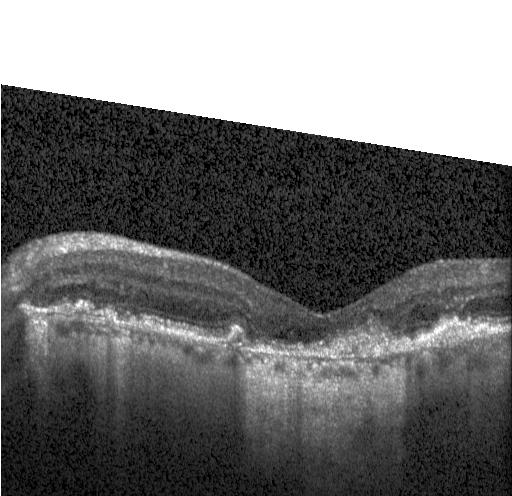

Retinal OCT cross-section · acquired on a Heidelberg Spectralis
The scan shows a choroidal neovascular membrane.